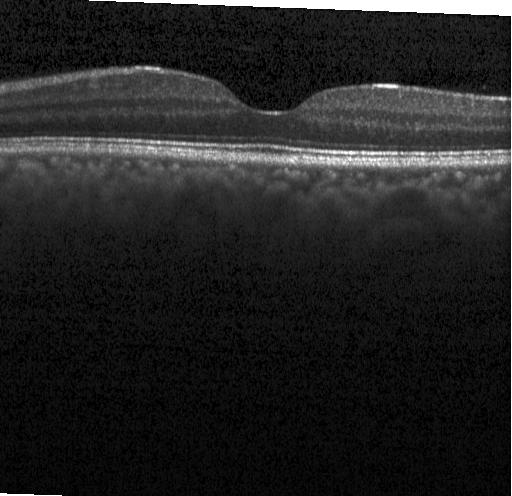
Diagnosis: neither choroidal neovascularization, diabetic macular edema, nor drusen.